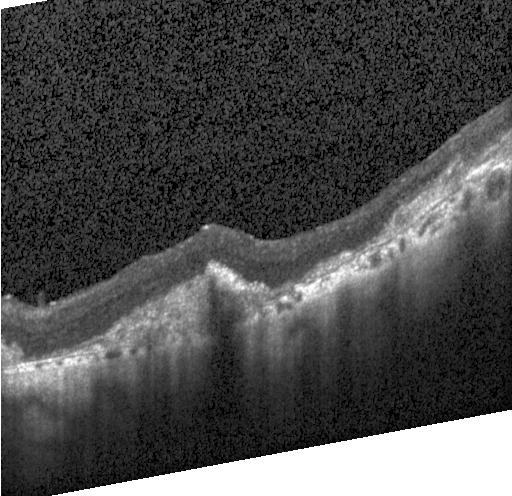 OCT B-scan showing a choroidal neovascular membrane.